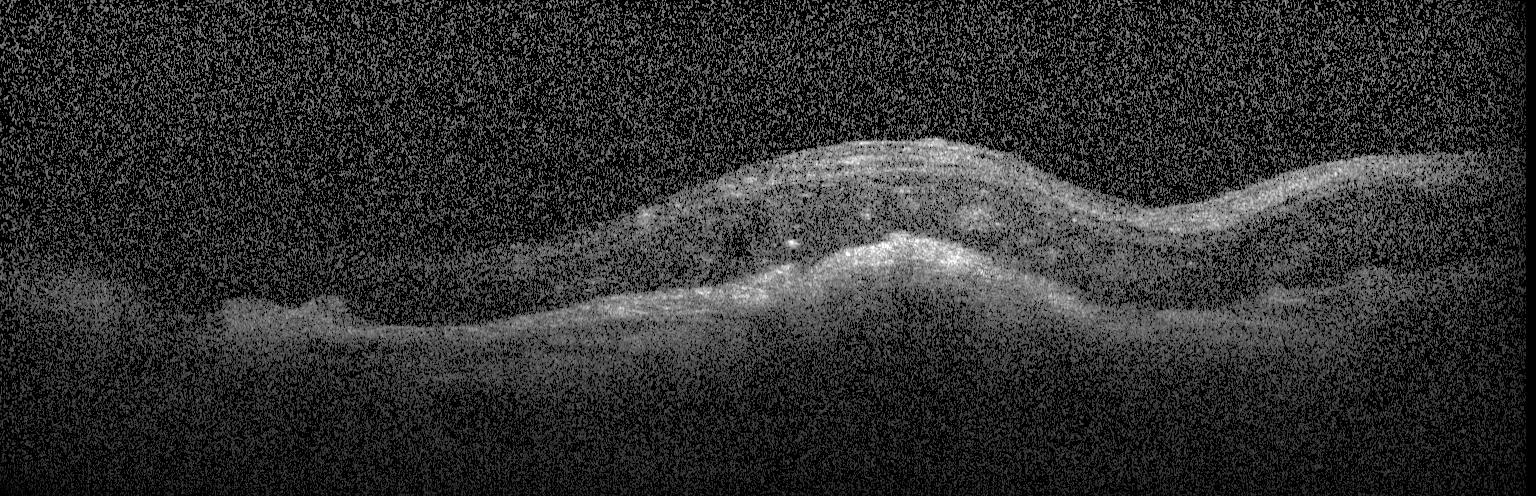

OCT B-scan, SD-OCT, macular scan, Heidelberg Spectralis OCT system. Impression: CNV.